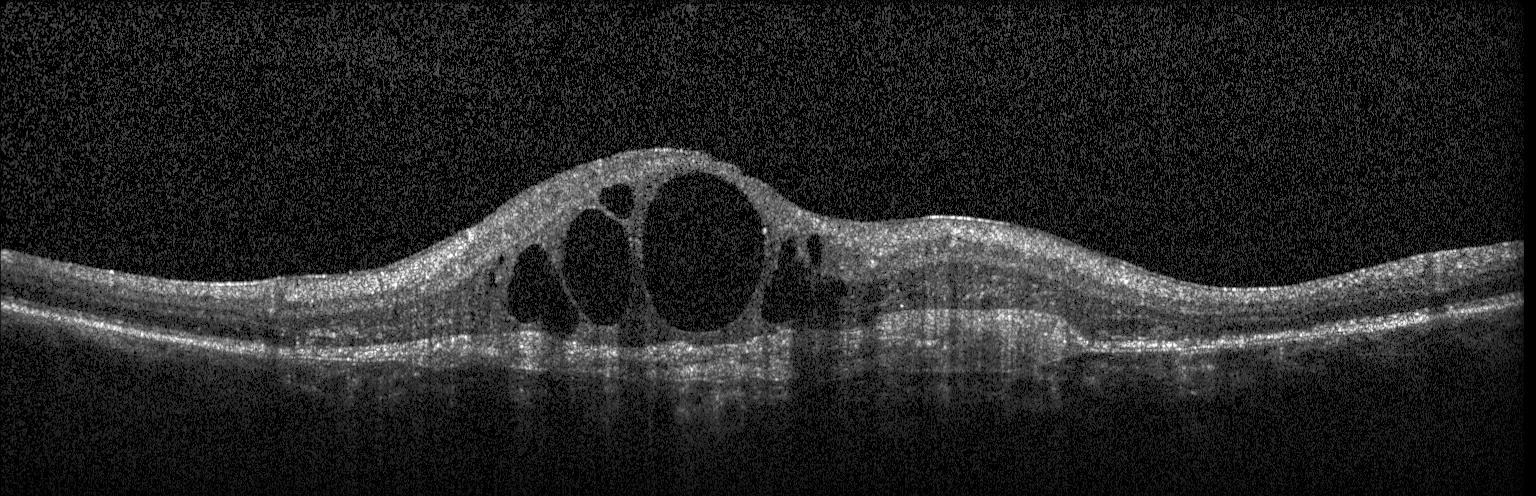
Spectral-domain OCT, centered on the fovea, OCT B-scan, instrument: Heidelberg Spectralis — A choroidal neovascular membrane.